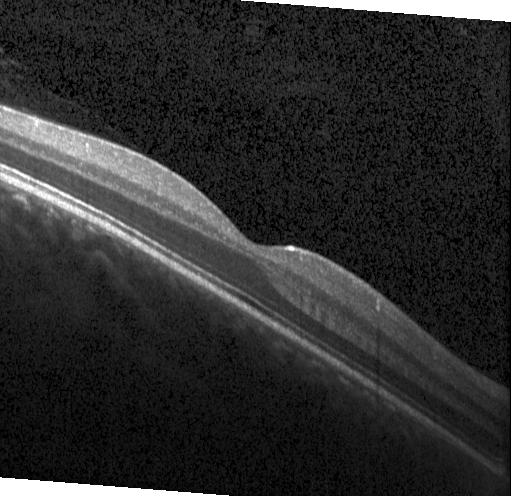 SD-OCT, Heidelberg Spectralis OCT system, optical coherence tomography B-scan, horizontal scan through the fovea.
This B-scan demonstrates no CNV, DME, or drusen.